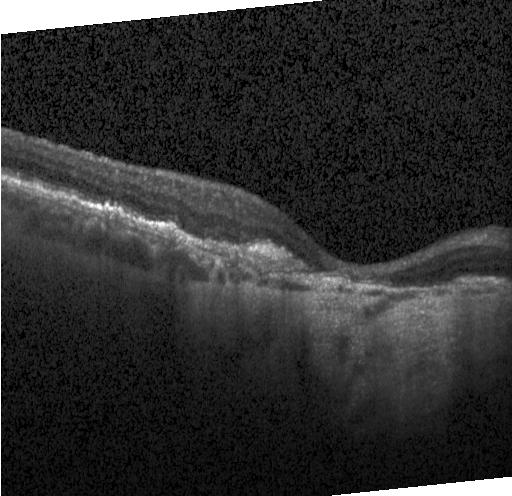

Spectral-domain optical coherence tomography; retinal OCT B-scan
Impression: choroidal neovascularization (CNV).